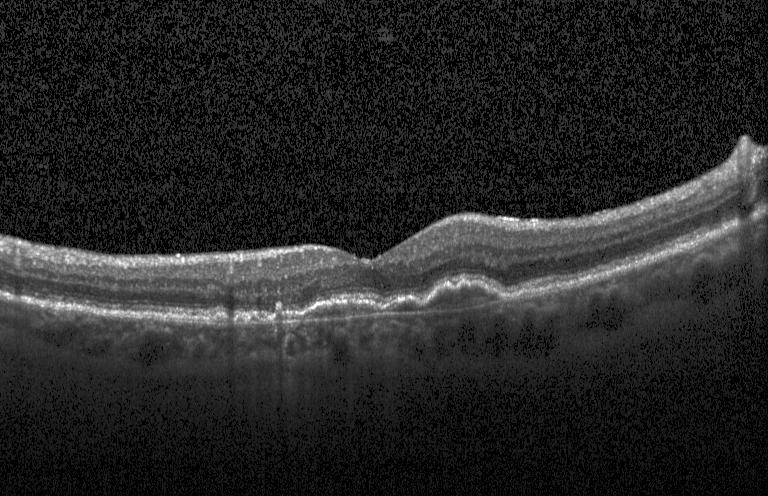 Macular scan. Optical coherence tomography scan. SD-OCT.
Diagnosis: choroidal neovascularization.